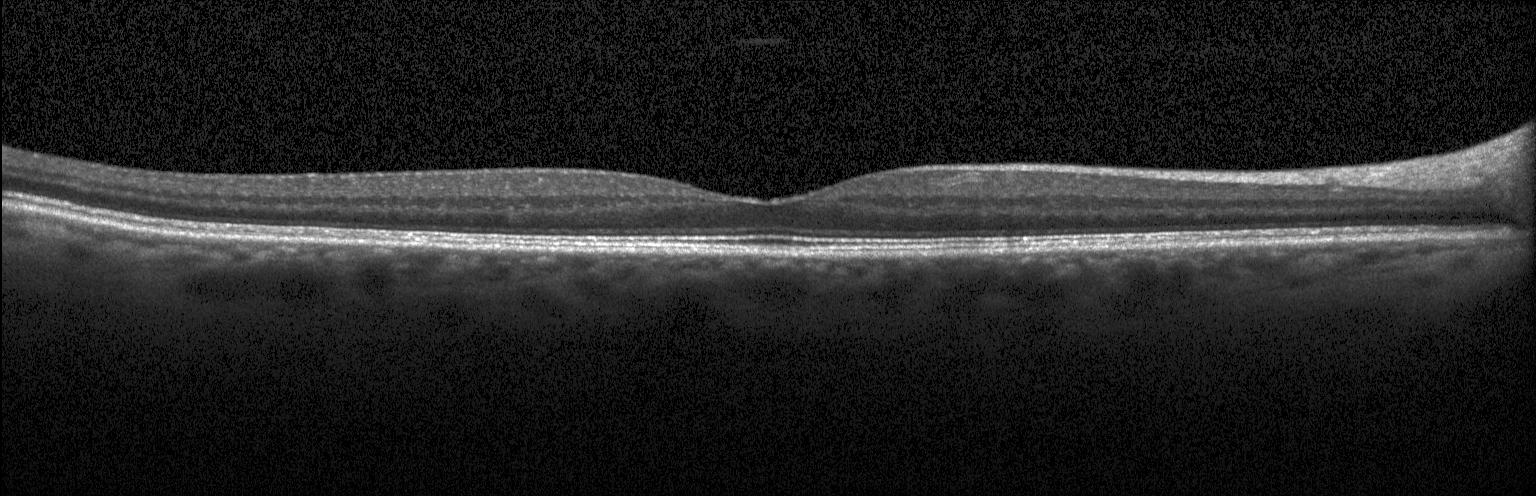 OCT B-scan; centered on the fovea; spectral-domain optical coherence tomography; Heidelberg Spectralis.
Assessment: neither CNV, DME, nor drusen.